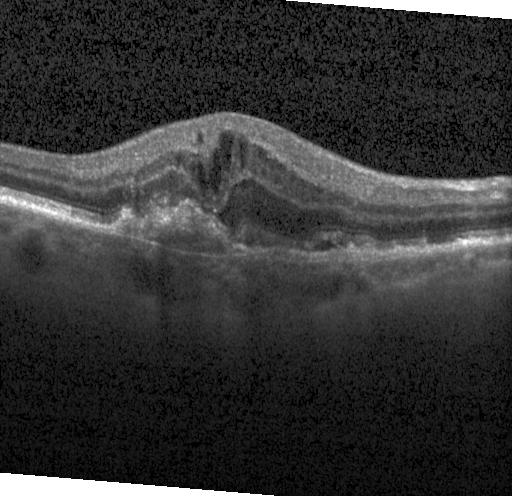
Through the macula, Heidelberg Spectralis OCT system, optical coherence tomography B-scan.
Finding: a choroidal neovascular membrane.